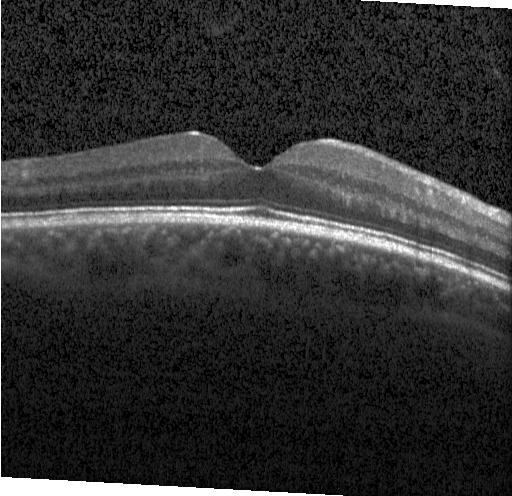

OCT line scan.
OCT finding: no choroidal neovascularization, diabetic macular edema, or drusen.